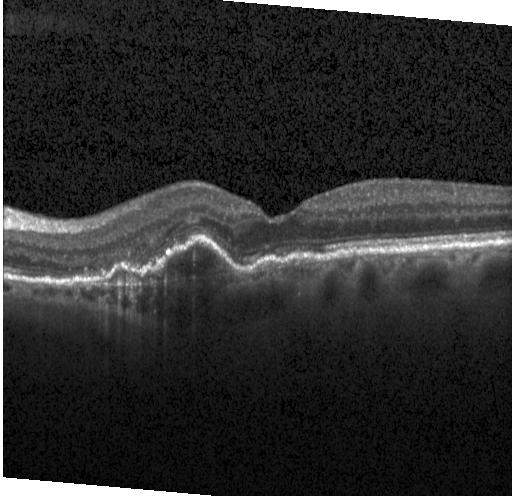

Retinal OCT cross-section
Diagnosis: a choroidal neovascular membrane.